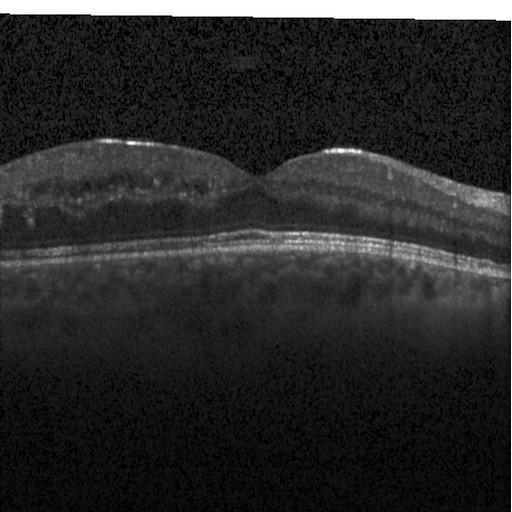 Optical coherence tomography B-scan. Instrument: Heidelberg Spectralis. Centered on the fovea — Assessment: diabetic macular edema.